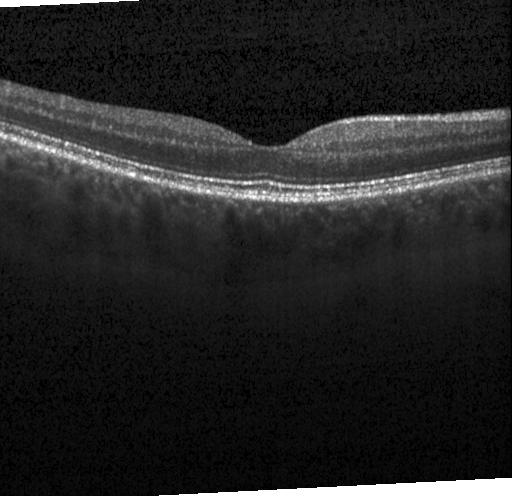

Spectral-domain OCT B-scan: no CNV, no DME, and no drusen.